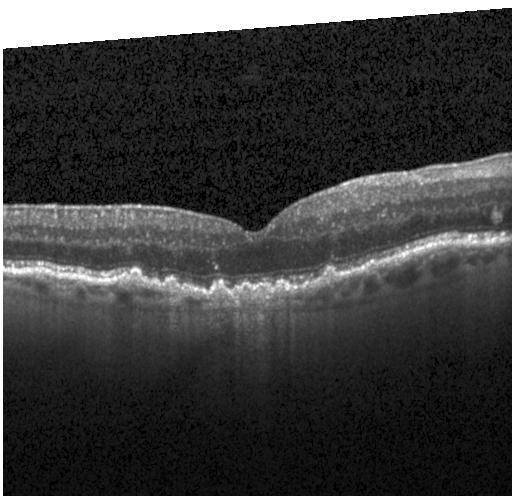

Spectral-domain OCT B-scan: a choroidal neovascular membrane.